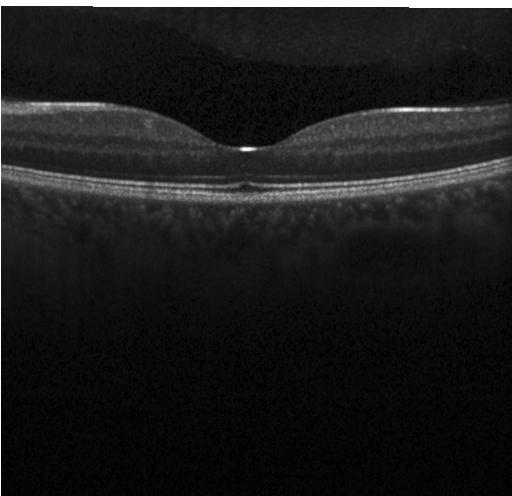

Finding: no evidence of choroidal neovascularization, diabetic macular edema, or drusen.